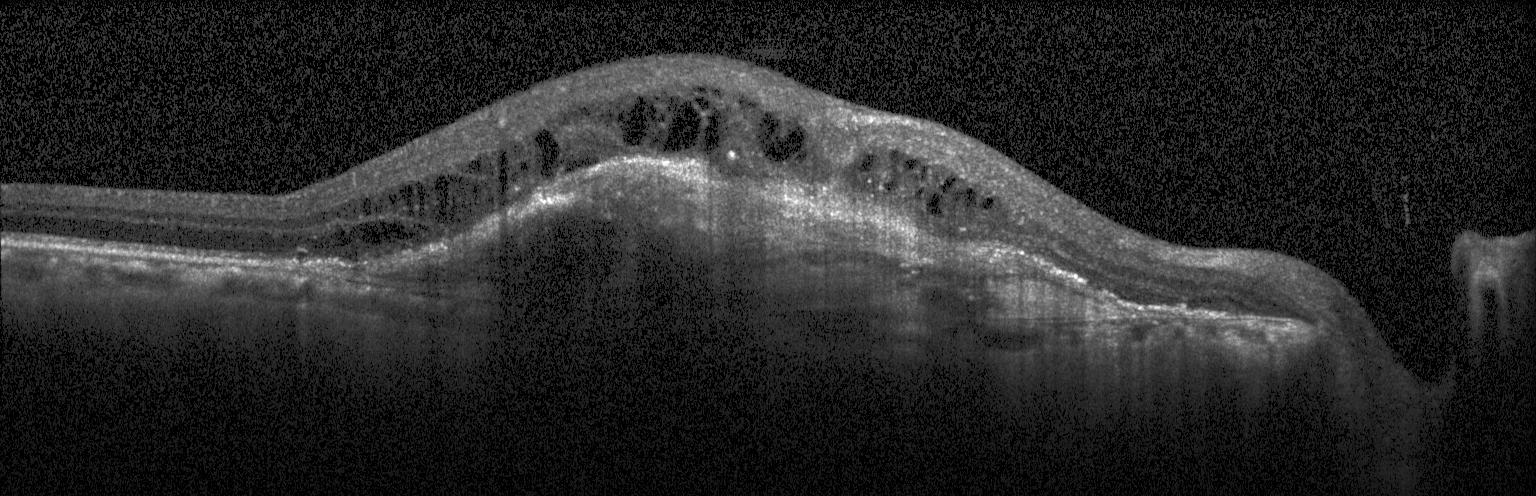

OCT line scan, Heidelberg Spectralis OCT system, SD-OCT — Finding: a choroidal neovascular membrane.